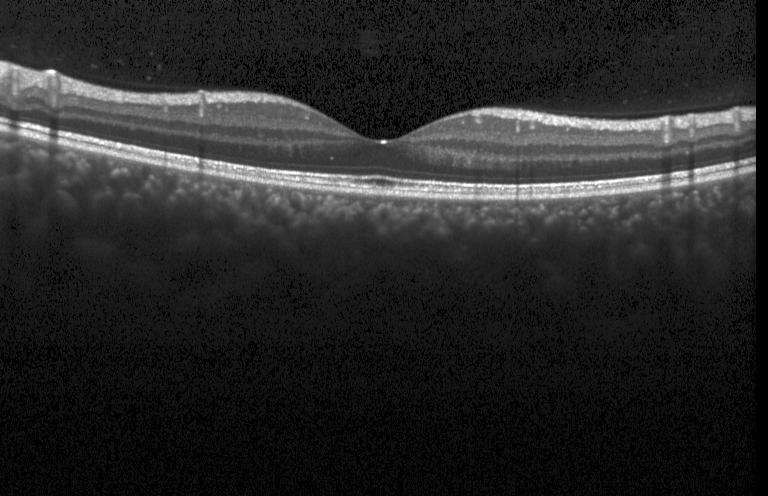

Heidelberg Spectralis OCT system; macular scan; retinal OCT B-scan. Finding: neither choroidal neovascularization, diabetic macular edema, nor drusen.